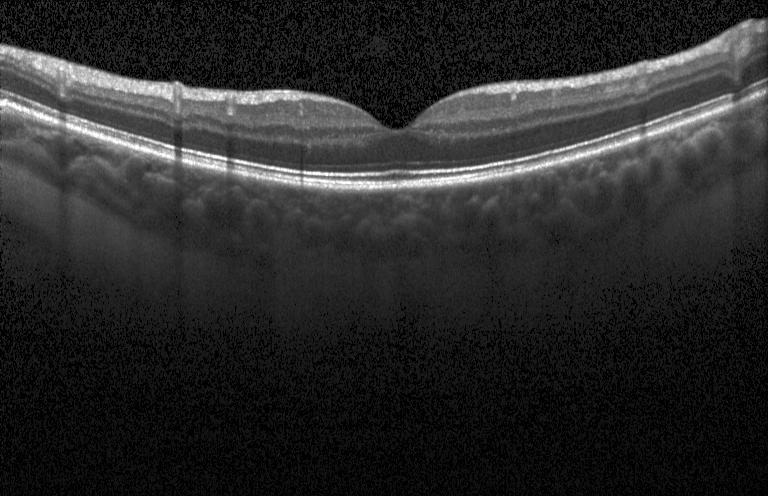 OCT line scan; horizontal scan through the fovea — No choroidal neovascularization, no diabetic macular edema, and no drusen.